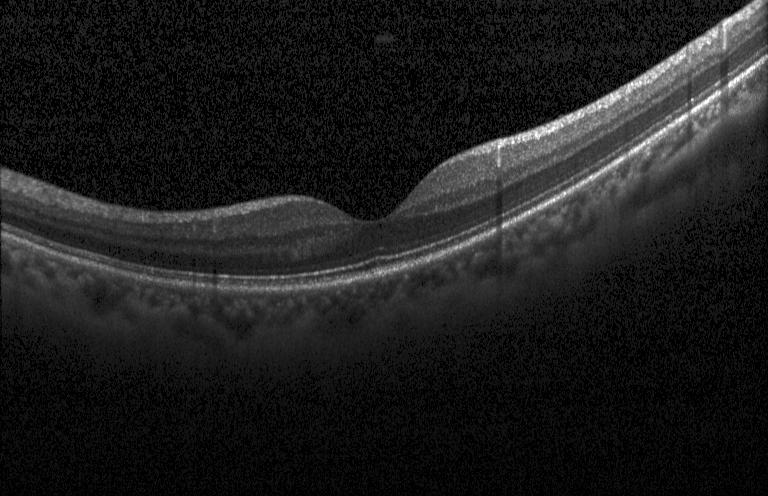

Heidelberg Spectralis · centered on the fovea · retinal OCT cross-section — Assessment: no evidence of choroidal neovascularization, diabetic macular edema, or drusen.